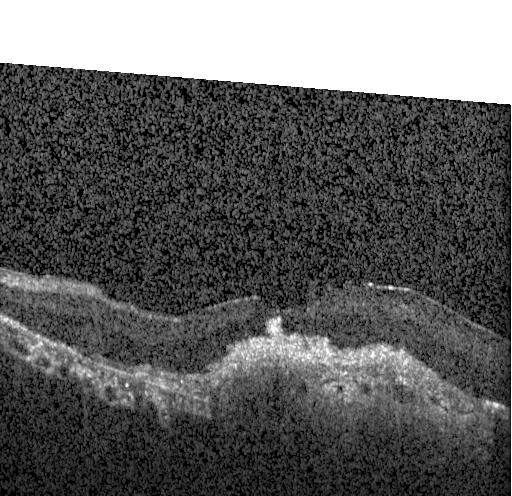 Impression: choroidal neovascularization.